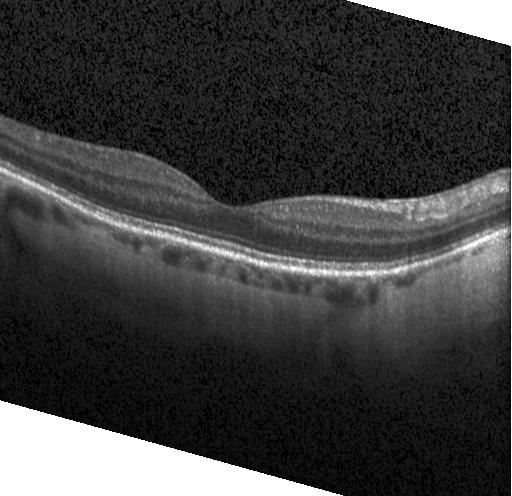
Optical coherence tomography B-scan
Diagnosis: no evidence of choroidal neovascularization, diabetic macular edema, or drusen.